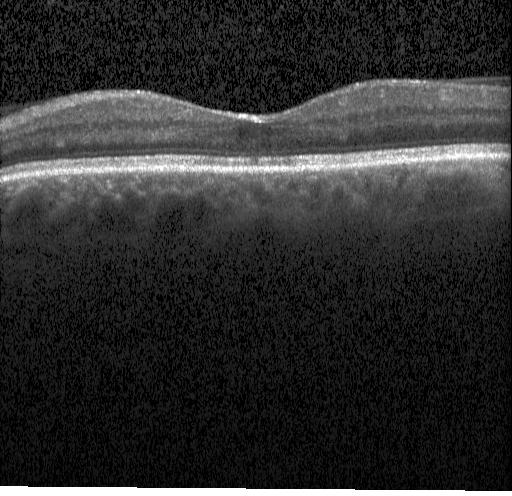

Diagnosis: no evidence of choroidal neovascularization, diabetic macular edema, or drusen.